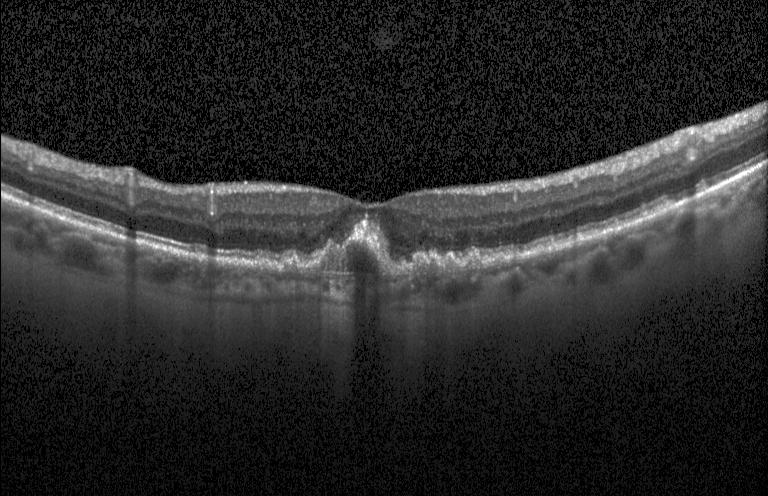 Retinal OCT cross-section. CNV.